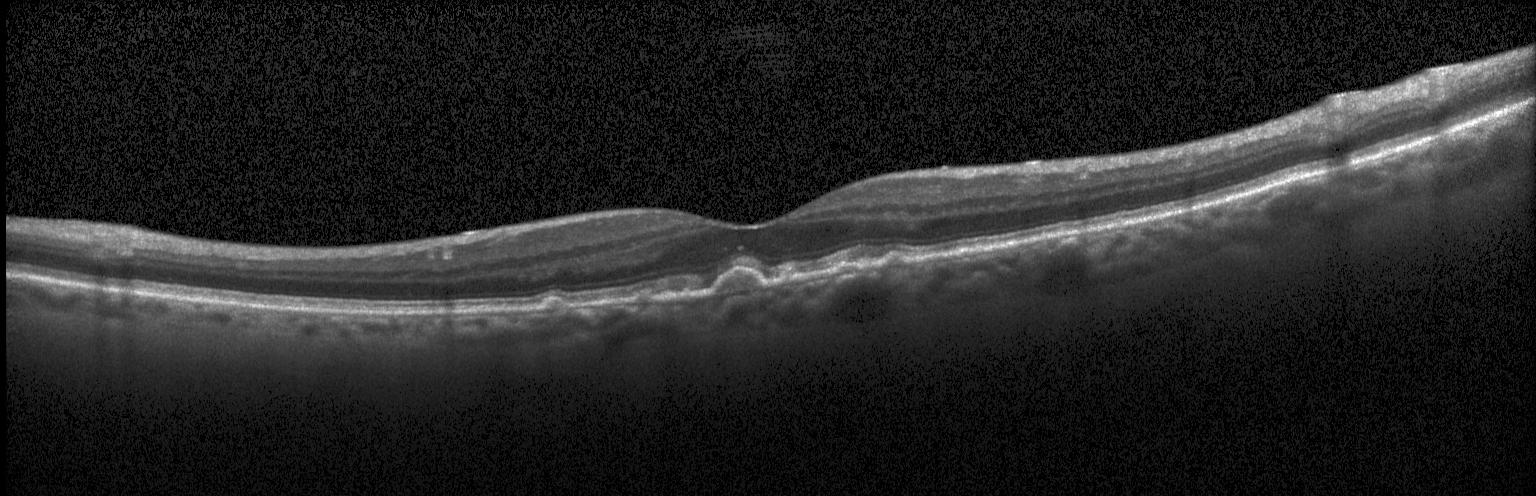

Spectral-domain OCT B-scan: drusen.